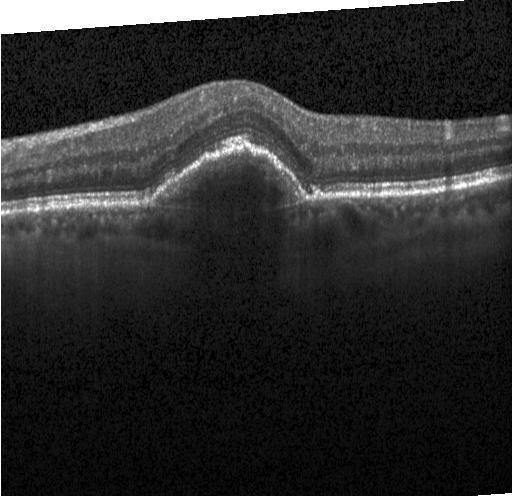

Retinal OCT cross-section showing a choroidal neovascular membrane.